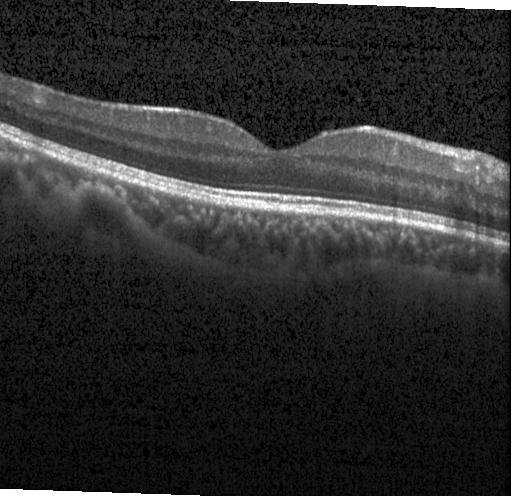 OCT B-scan · SD-OCT · Heidelberg Spectralis
OCT finding: no choroidal neovascularization, no diabetic macular edema, and no drusen.